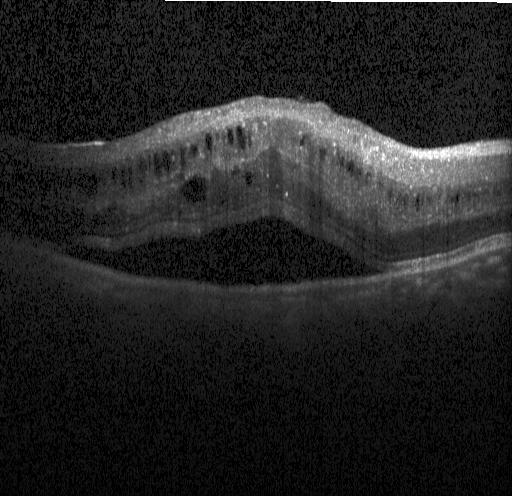

Fovea-centered, retinal OCT B-scan, spectral-domain optical coherence tomography. Finding: diabetic macular edema.